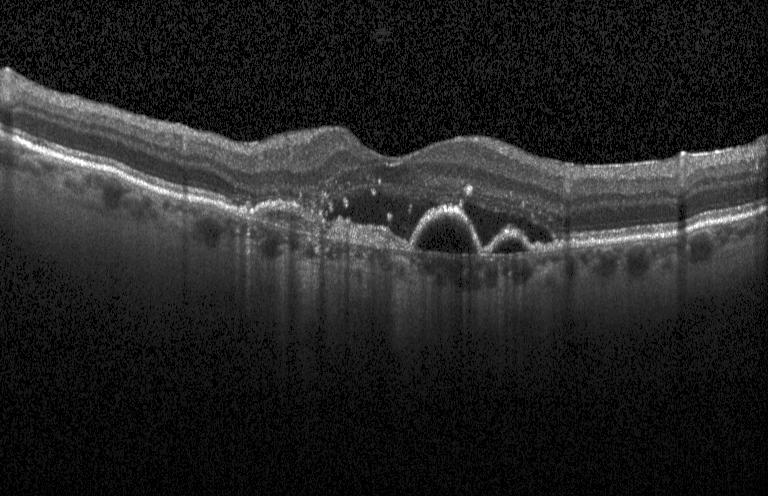
Impression: CNV.